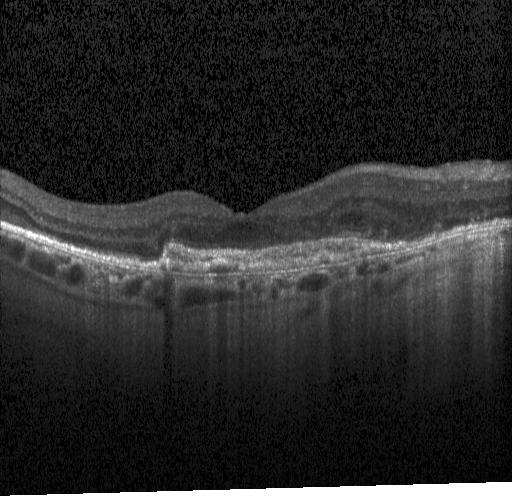
Impression: choroidal neovascularization.